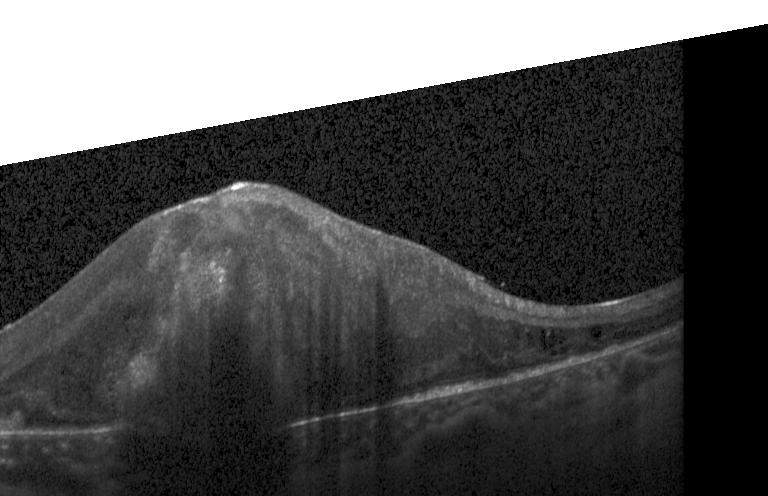
Impression: choroidal neovascularization.